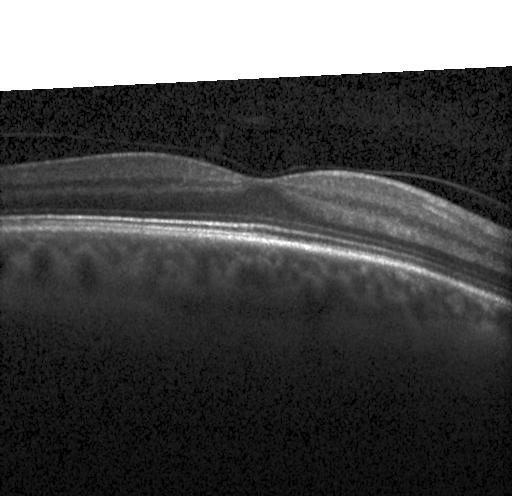
Optical coherence tomography B-scan.
This B-scan demonstrates no evidence of CNV, DME, or drusen.